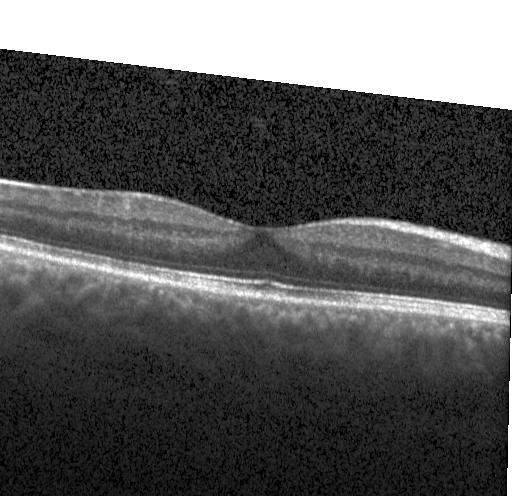

OCT scan showing neither CNV, DME, nor drusen.